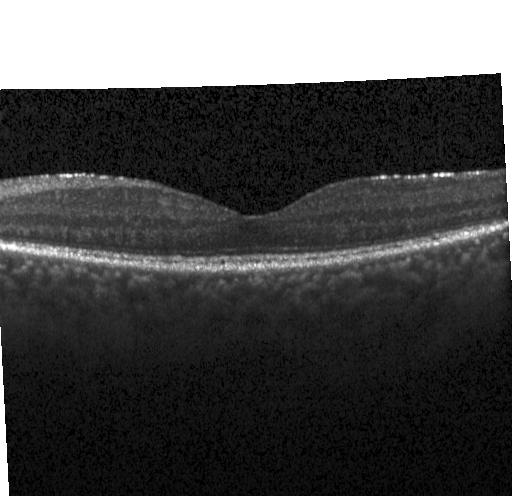

Optical coherence tomography scan, instrument: Heidelberg Spectralis
Dx: no CNV, DME, or drusen.